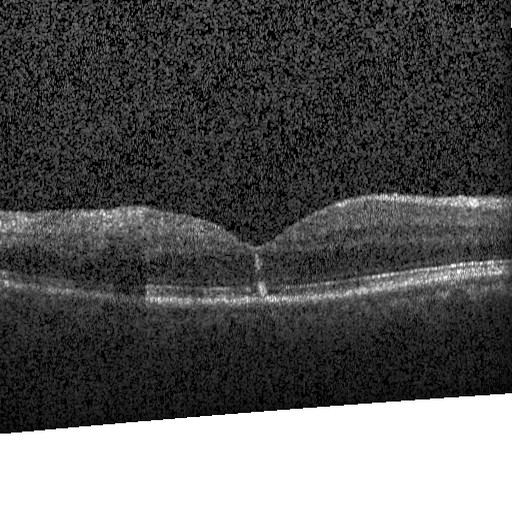

Diabetic macular edema.